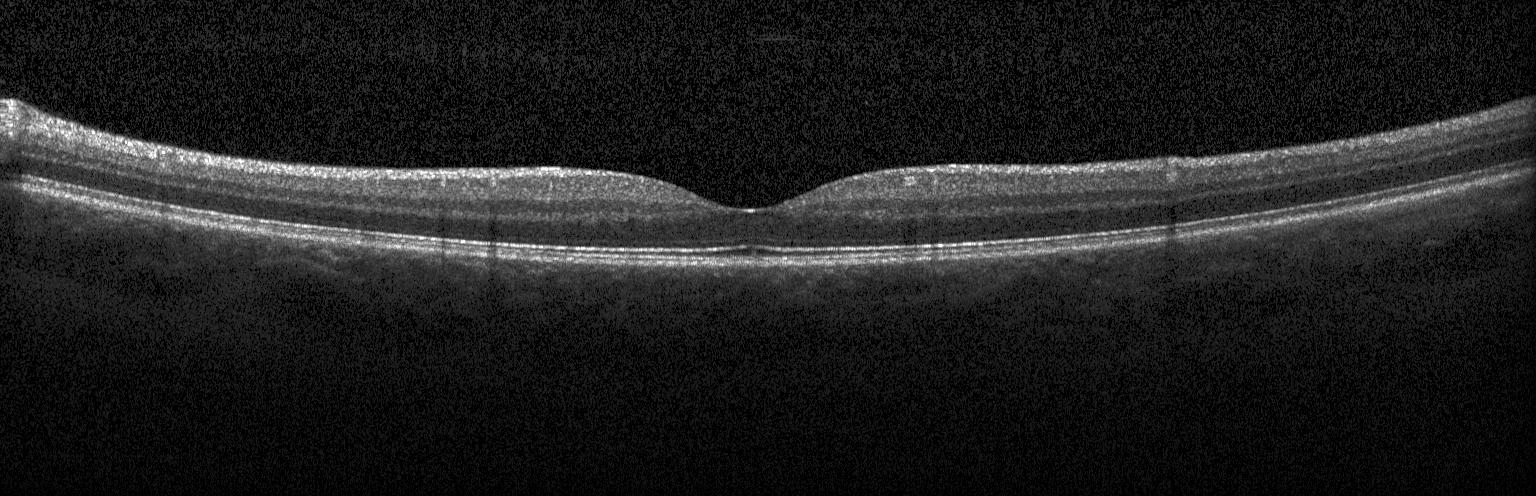 Retinal OCT B-scan. Dx: neither choroidal neovascularization, diabetic macular edema, nor drusen.